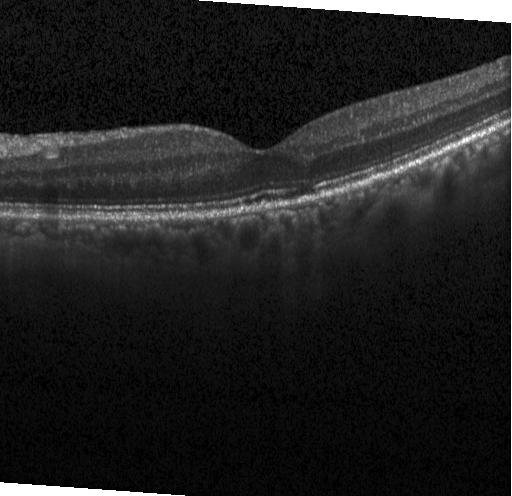
Acquired on a Heidelberg Spectralis; fovea-centered; OCT B-scan. Dx: no choroidal neovascularization, no diabetic macular edema, and no drusen.